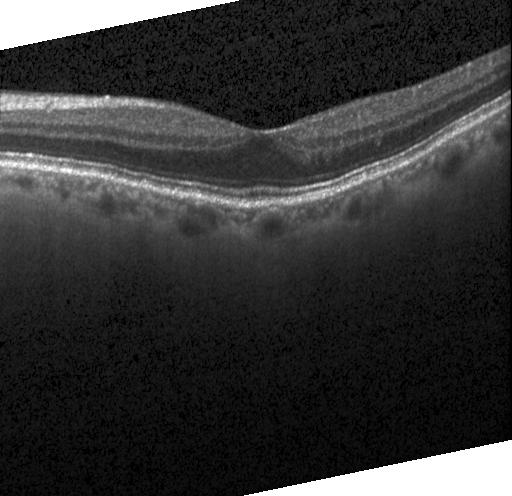

OCT B-scan. Heidelberg Spectralis OCT system. Spectral-domain OCT
No CNV, no DME, and no drusen.